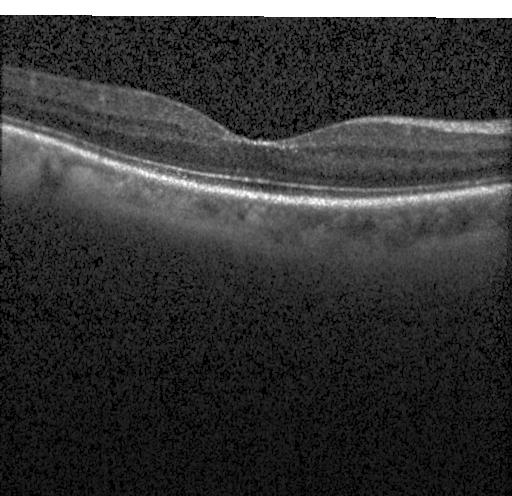

Fovea-centered, instrument: Heidelberg Spectralis, optical coherence tomography scan — Finding: no evidence of choroidal neovascularization, diabetic macular edema, or drusen.